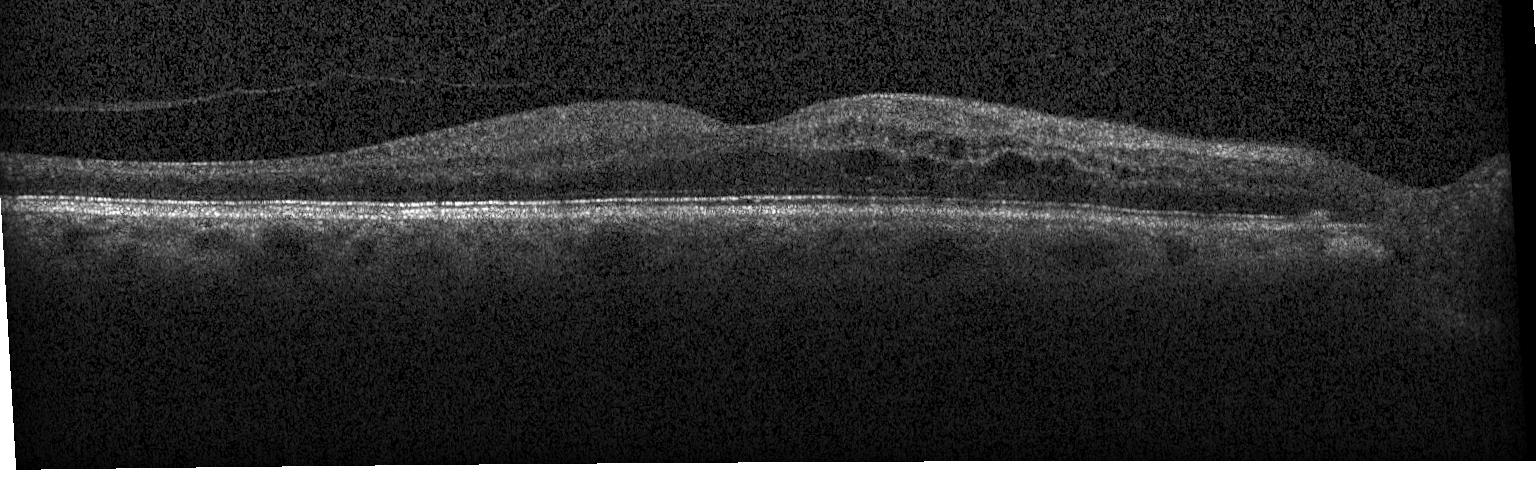
Diabetic macular edema.